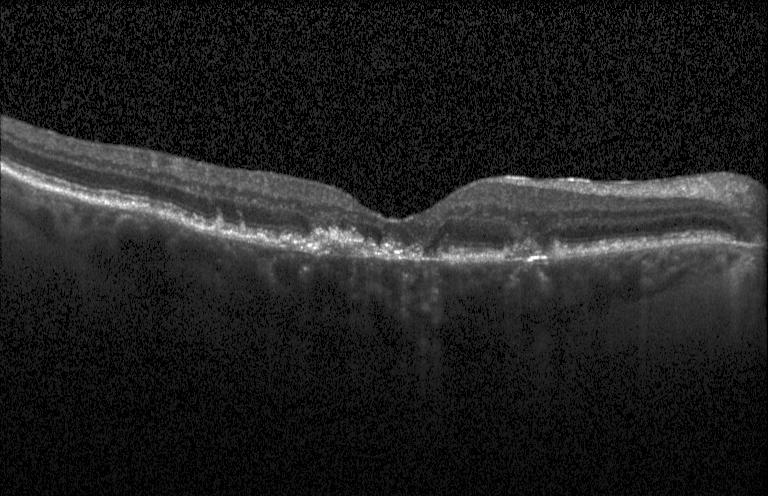 Heidelberg Spectralis. Spectral-domain optical coherence tomography. Fovea-centered. Optical coherence tomography B-scan. Assessment: a choroidal neovascular membrane.